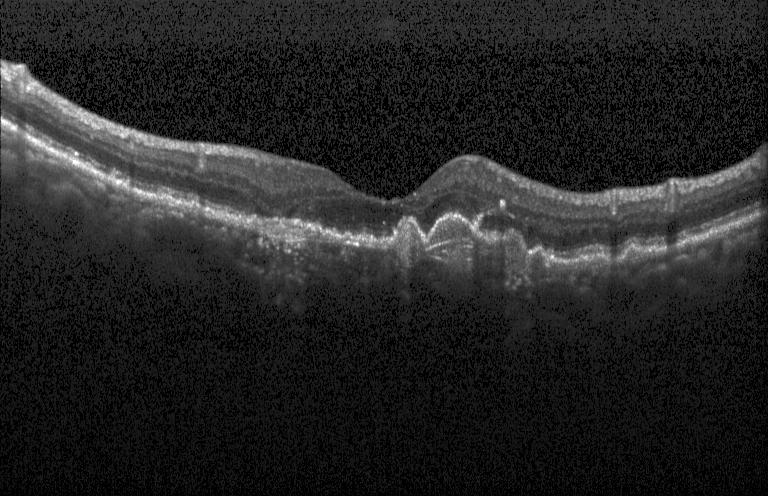

SD-OCT, OCT B-scan. Finding: choroidal neovascularization (CNV).